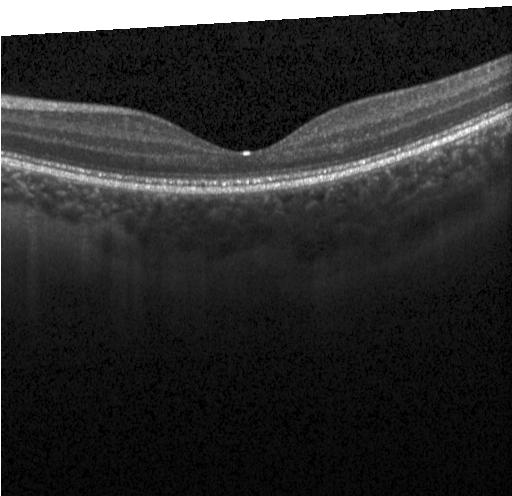
Retinal OCT B-scan · fovea-centered — Impression: no choroidal neovascularization, no diabetic macular edema, and no drusen.